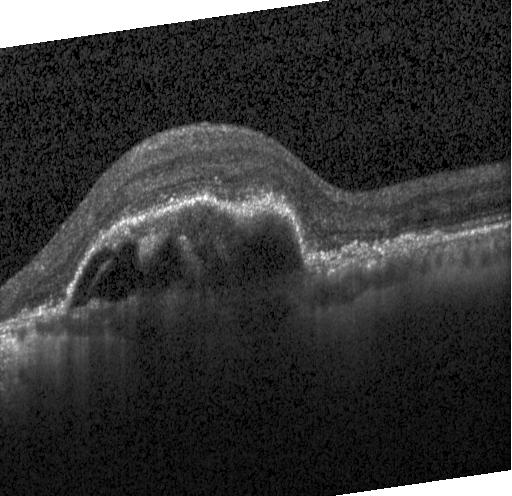

Macular OCT demonstrating CNV.